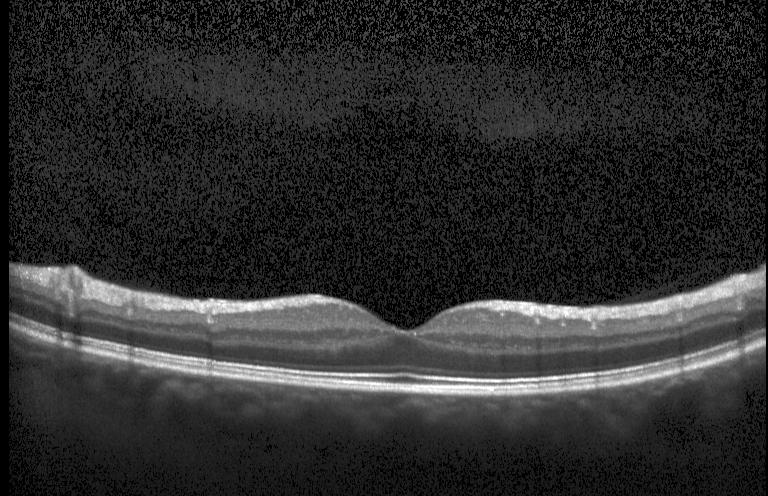

Centered on the fovea, spectral-domain OCT, retinal OCT cross-section. Finding: no choroidal neovascularization, diabetic macular edema, or drusen.